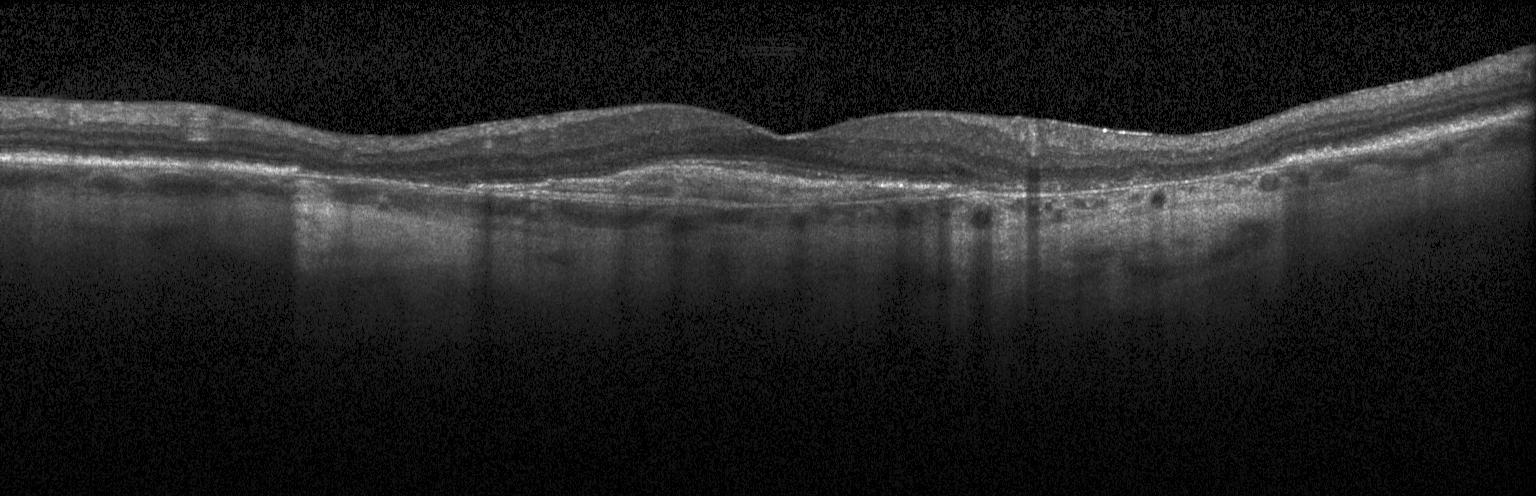
Retinal OCT B-scan
The scan shows a choroidal neovascular membrane.